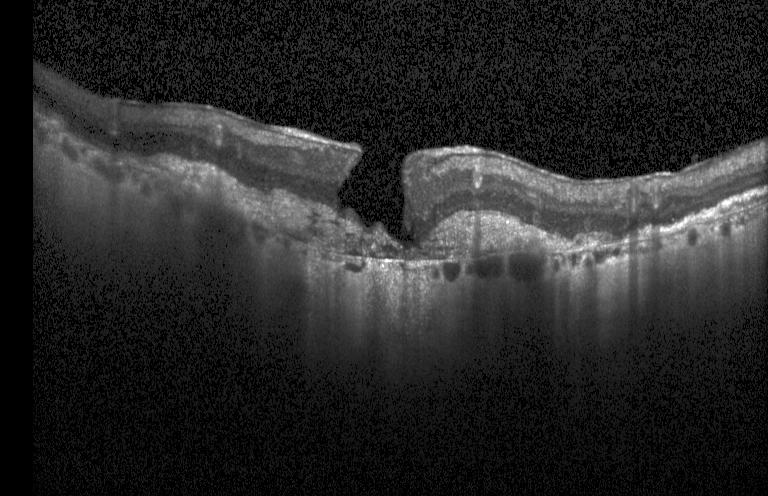
Retinal OCT cross-section, fovea-centered, Heidelberg Spectralis OCT system.
Impression: CNV.